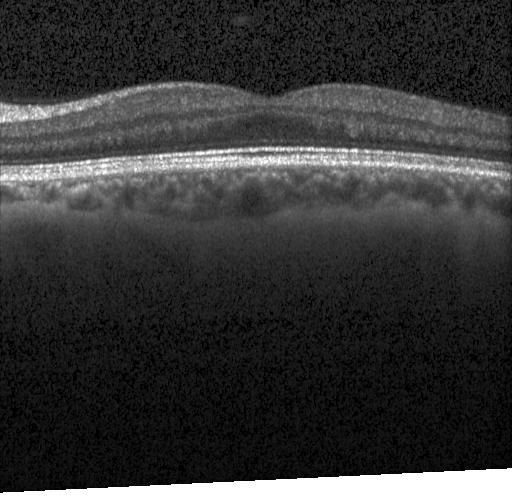 Retinal OCT B-scan. Finding: no evidence of CNV, DME, or drusen.